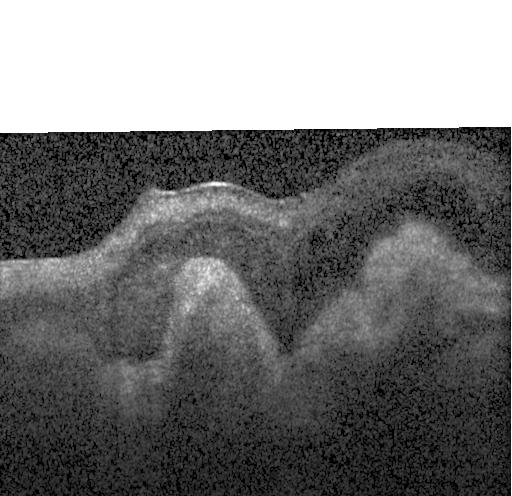
Impression: choroidal neovascularization.